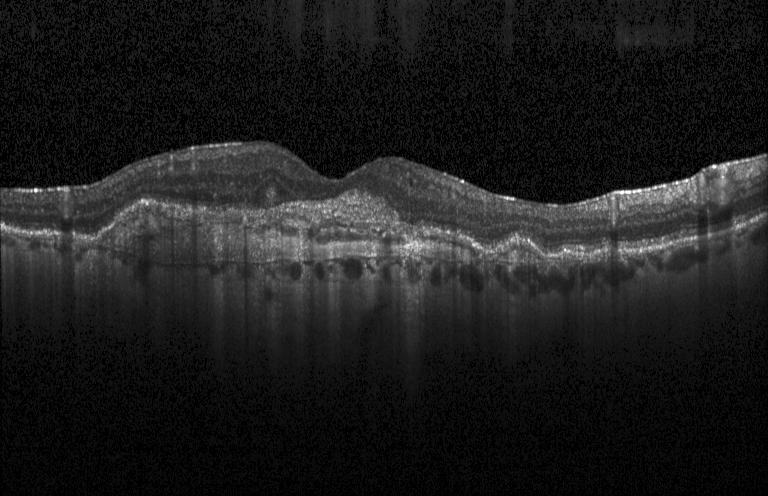 Retinal OCT B-scan; SD-OCT
Diagnosis: a choroidal neovascular membrane.